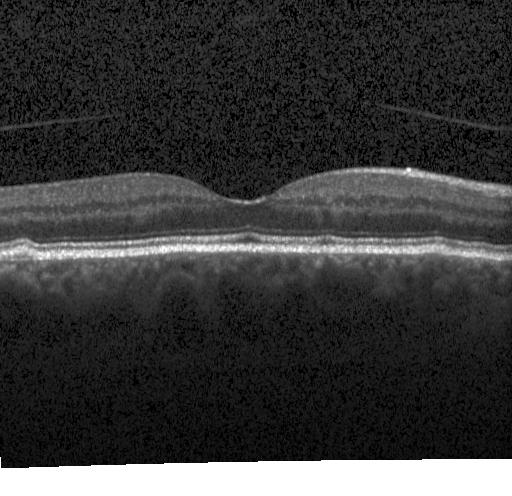
Retinal OCT B-scan — The scan shows sub-RPE drusenoid deposits.